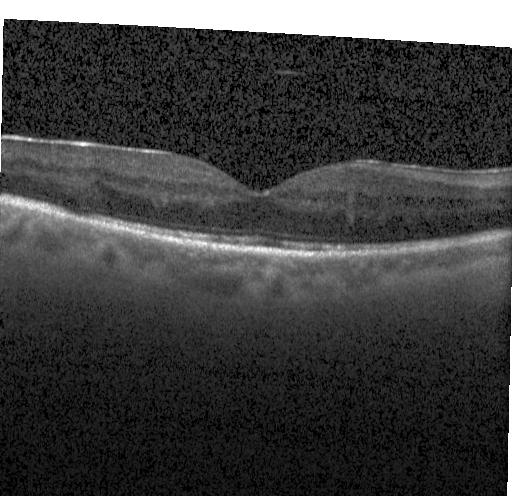
OCT B-scan. Finding: neither CNV, DME, nor drusen.